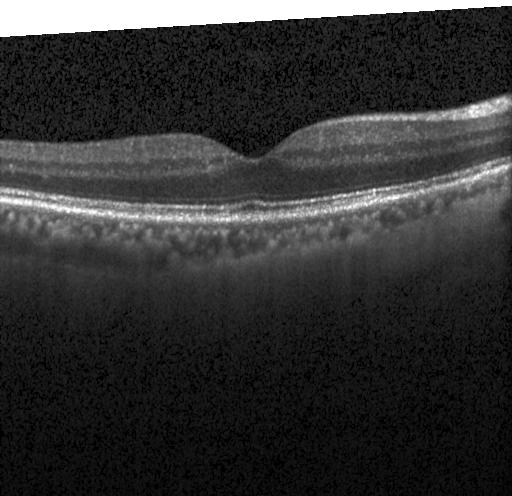
OCT finding: no choroidal neovascularization, no diabetic macular edema, and no drusen.